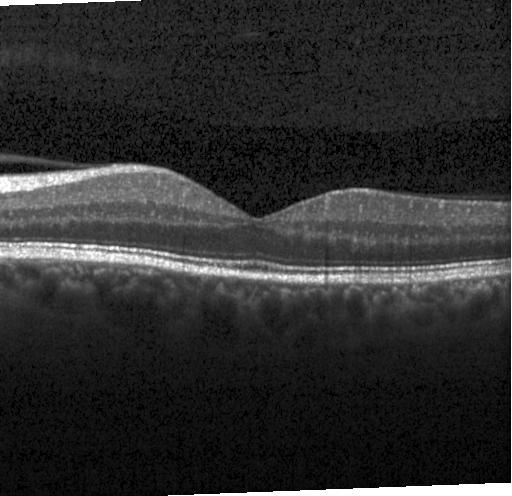
OCT B-scan; Heidelberg Spectralis OCT system; SD-OCT — Diagnosis: no choroidal neovascularization, no diabetic macular edema, and no drusen.